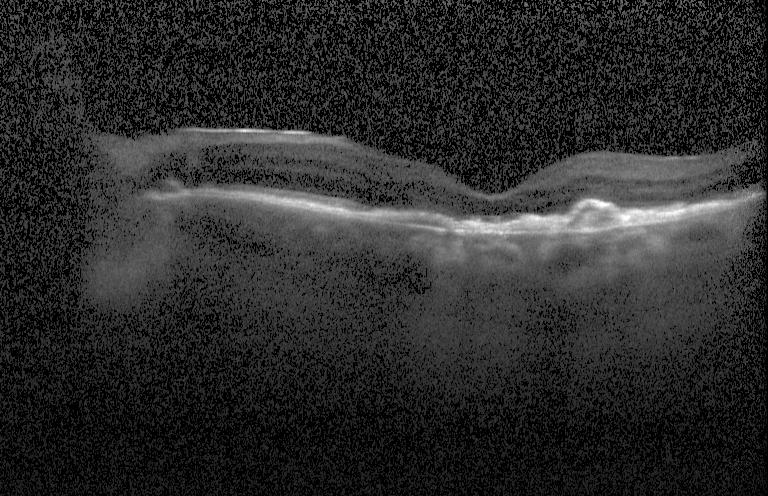 Macular OCT: a choroidal neovascular membrane.